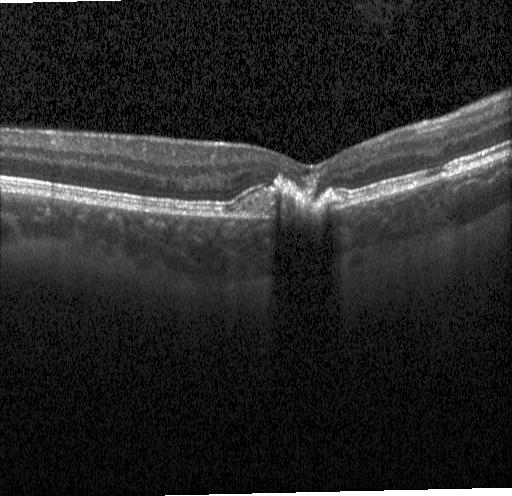 OCT B-scan — Finding: CNV.